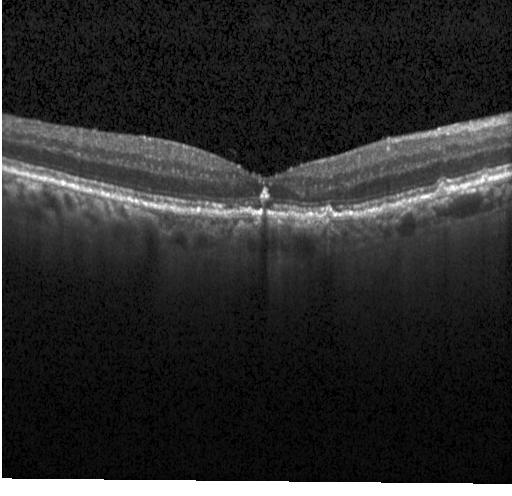

OCT B-scan. Centered on the fovea. Heidelberg Spectralis
Macular OCT: sub-RPE drusenoid deposits.